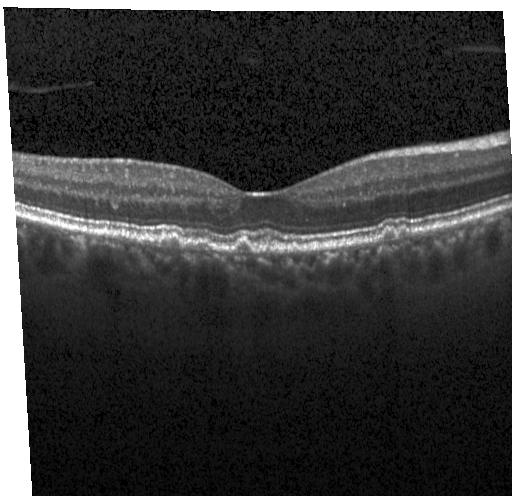 Optical coherence tomography scan.
Impression: drusen.